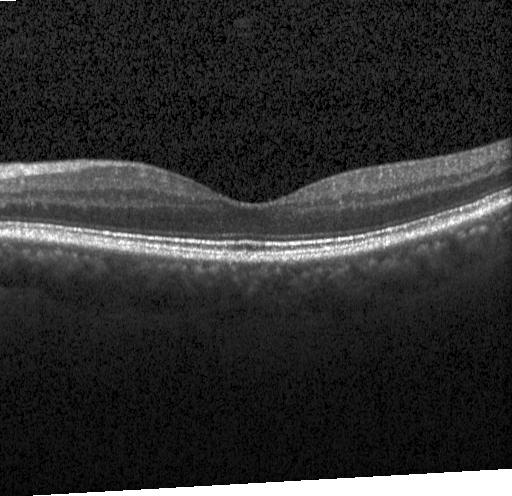

Retinal OCT B-scan.
This B-scan demonstrates no evidence of choroidal neovascularization, diabetic macular edema, or drusen.